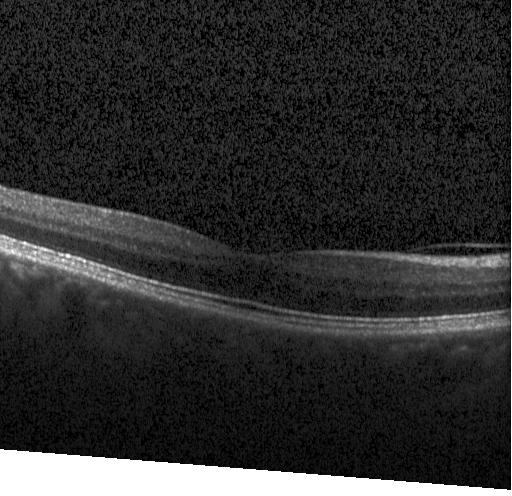 Macular scan · retinal OCT B-scan · SD-OCT · Heidelberg Spectralis OCT system.
The scan shows no choroidal neovascularization, no diabetic macular edema, and no drusen.